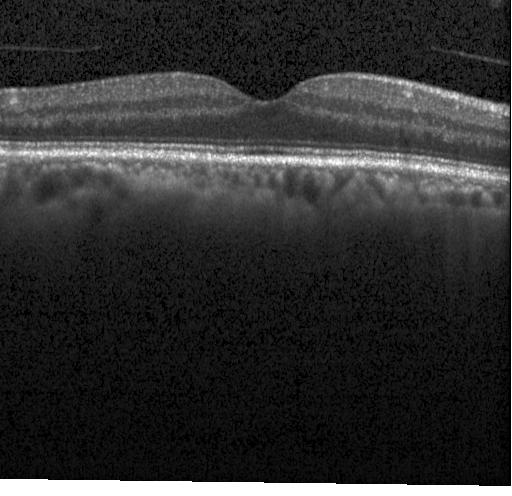
Centered on the fovea, instrument: Heidelberg Spectralis, spectral-domain optical coherence tomography, OCT line scan — Dx: no evidence of choroidal neovascularization, diabetic macular edema, or drusen.